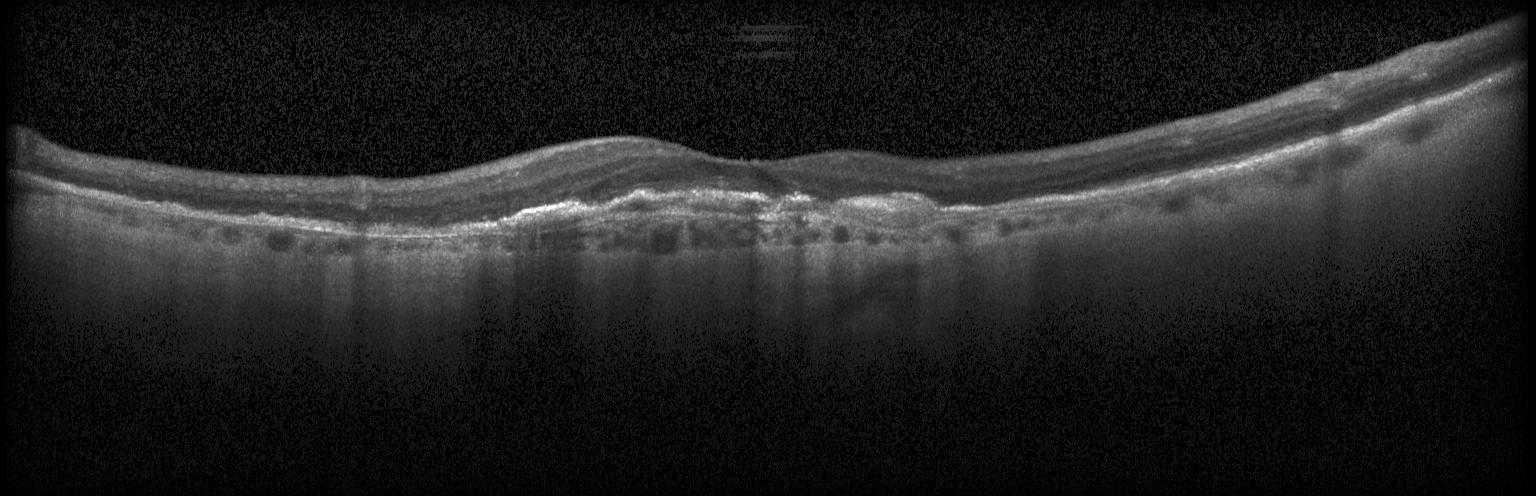 Impression: choroidal neovascularization.